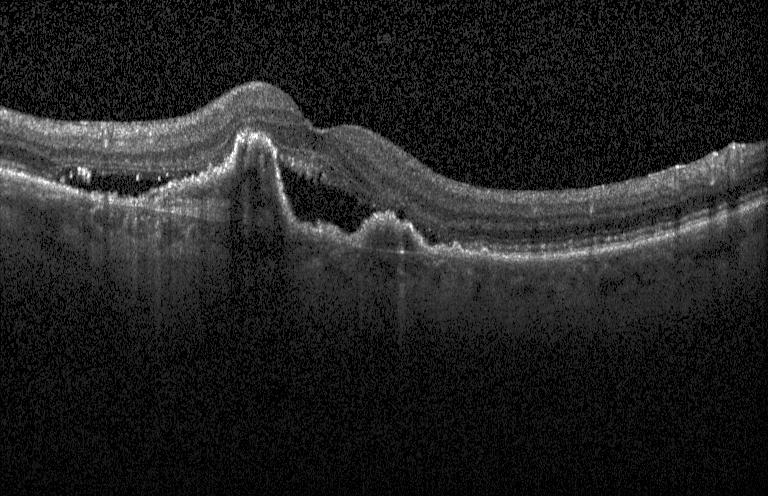

Through the macula · OCT B-scan · SD-OCT.
Dx: a choroidal neovascular membrane.